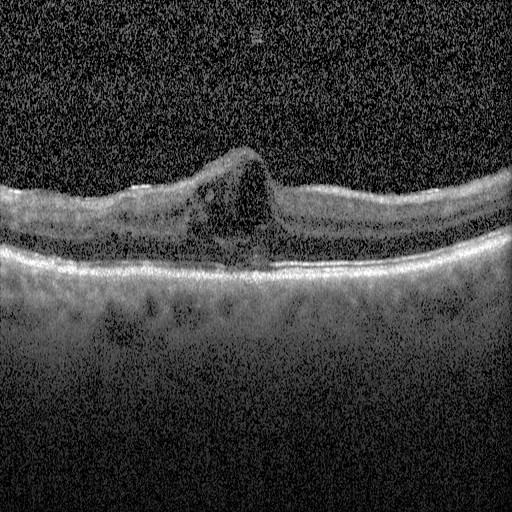 Diabetic macular edema.